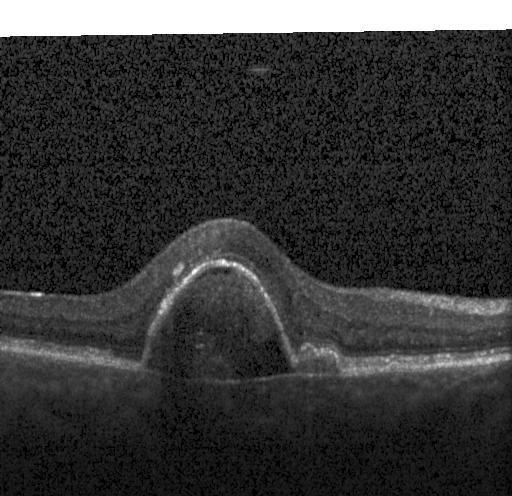

Diagnosis: choroidal neovascularization.